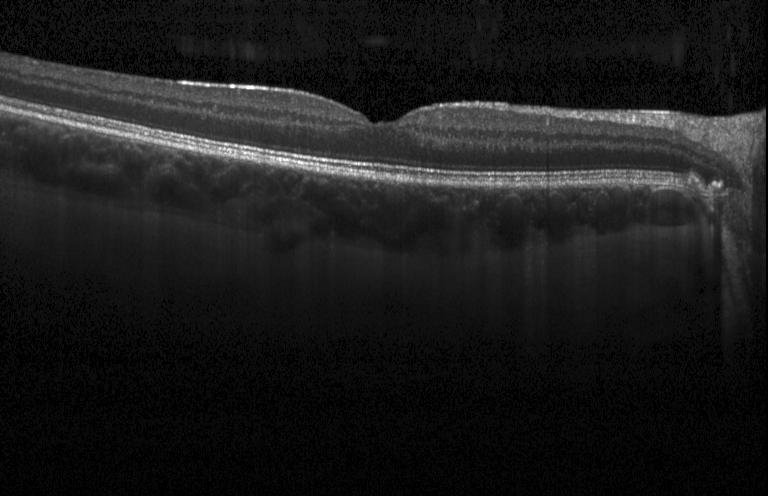
Diagnosis: no choroidal neovascularization, diabetic macular edema, or drusen.